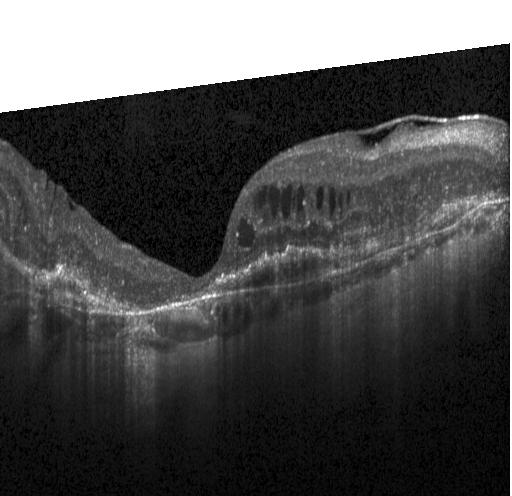
OCT B-scan, acquired on a Heidelberg Spectralis, spectral-domain OCT, fovea-centered. Finding: a choroidal neovascular membrane.